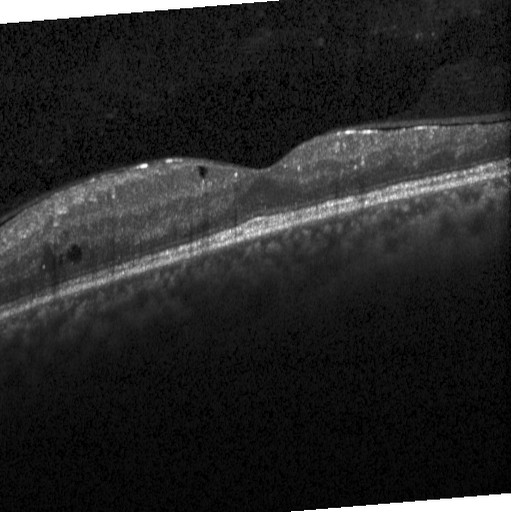

SD-OCT · retinal OCT cross-section · fovea-centered.
OCT finding: DME.